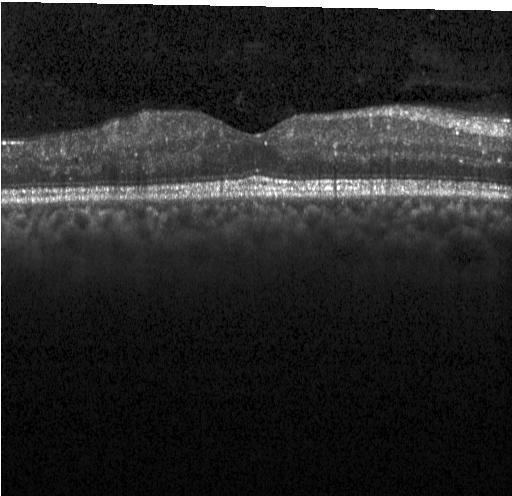

Spectral-domain optical coherence tomography, optical coherence tomography scan, macular scan, Heidelberg Spectralis OCT system.
Dx: DME.